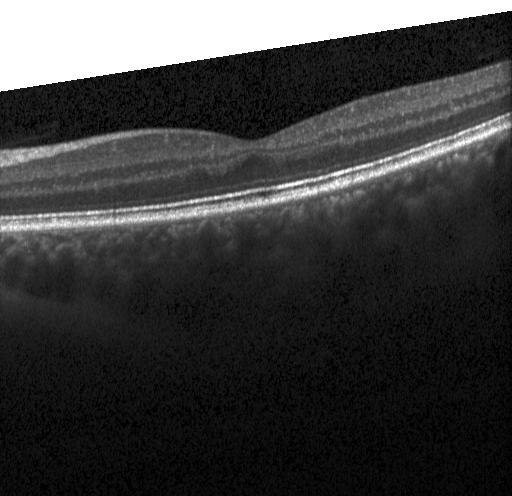 OCT B-scan. Spectral-domain OCT. Instrument: Heidelberg Spectralis
Impression: no CNV, no DME, and no drusen.